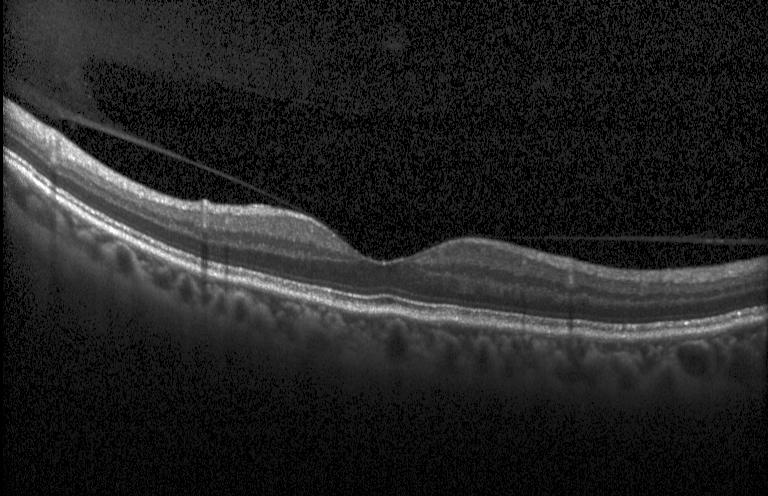

OCT B-scan; macular scan; SD-OCT; instrument: Heidelberg Spectralis.
Macular OCT: neither choroidal neovascularization, diabetic macular edema, nor drusen.